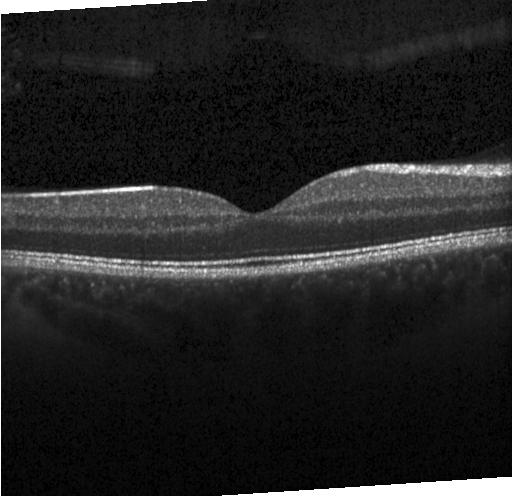
The scan shows neither CNV, DME, nor drusen.